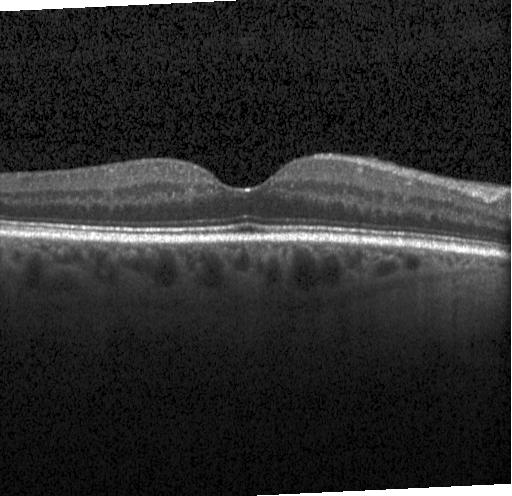

OCT B-scan
Diagnosis: neither choroidal neovascularization, diabetic macular edema, nor drusen.